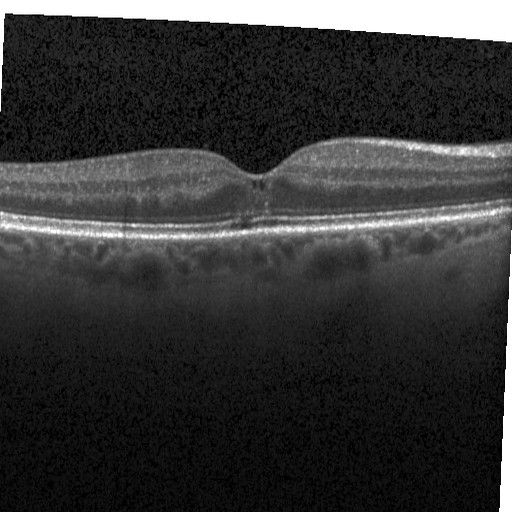

The scan shows diabetic macular edema.